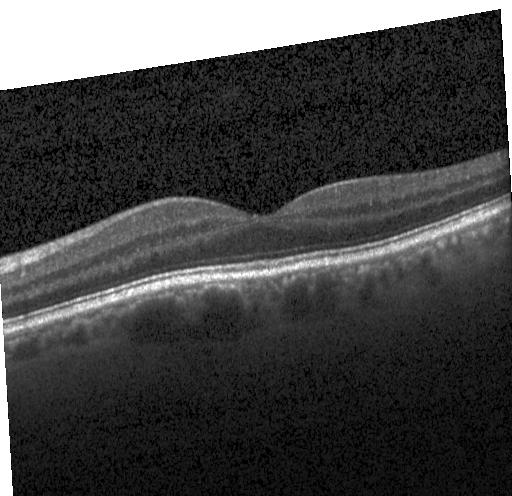

Heidelberg Spectralis OCT system, SD-OCT, OCT B-scan. Assessment: no choroidal neovascularization, diabetic macular edema, or drusen.